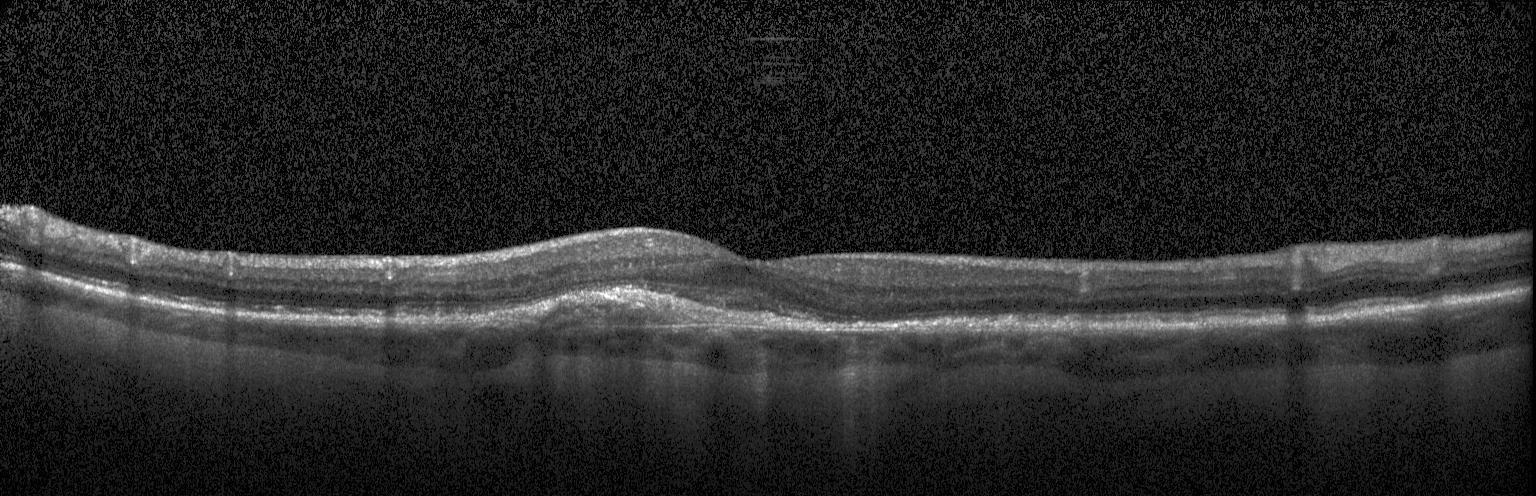 Finding: a choroidal neovascular membrane.